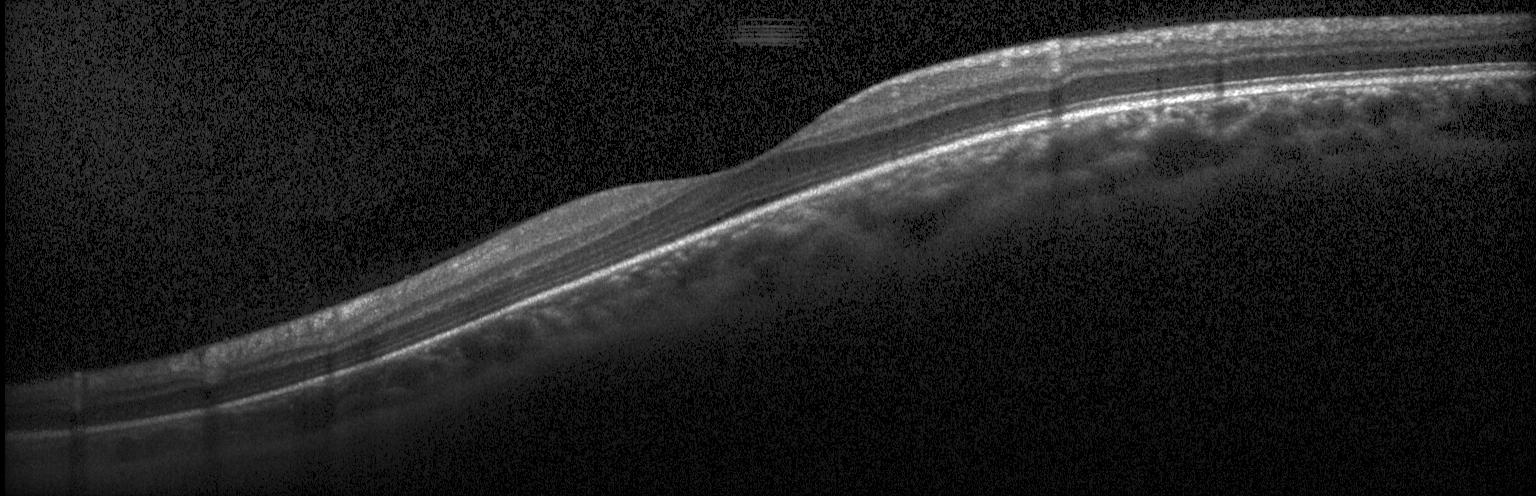

Retinal OCT B-scan — Finding: no evidence of CNV, DME, or drusen.